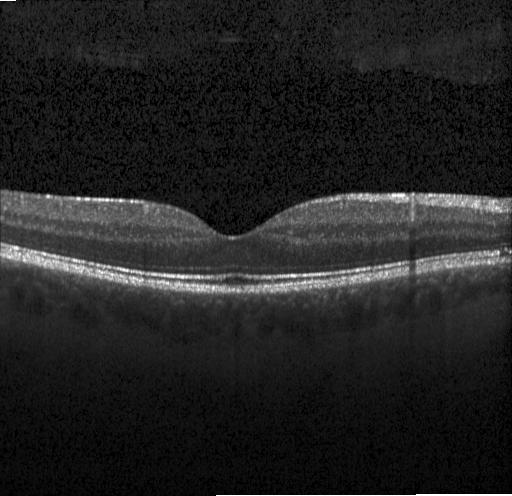 OCT B-scan.
Macular OCT: no evidence of choroidal neovascularization, diabetic macular edema, or drusen.